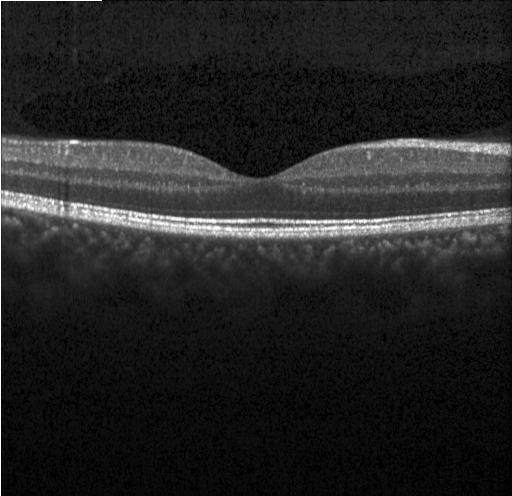 SD-OCT; retinal OCT B-scan — Dx: no choroidal neovascularization, diabetic macular edema, or drusen.